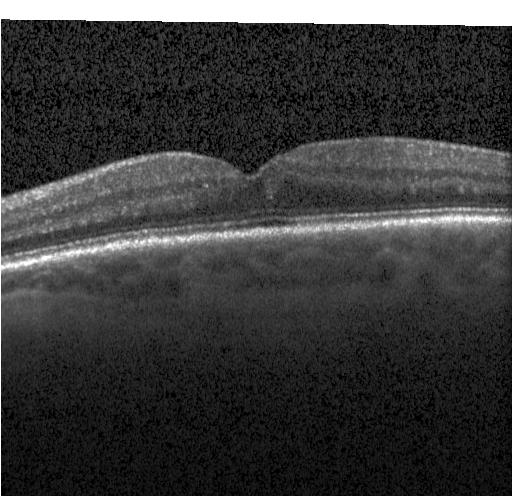
SD-OCT, OCT line scan — Impression: no choroidal neovascularization, no diabetic macular edema, and no drusen.